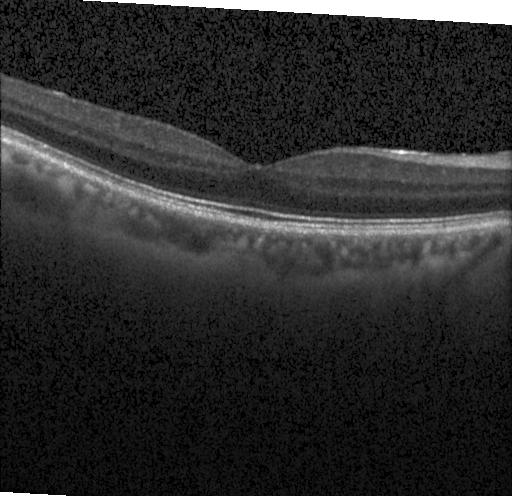
OCT B-scan. Heidelberg Spectralis.
Diagnosis: no evidence of choroidal neovascularization, diabetic macular edema, or drusen.